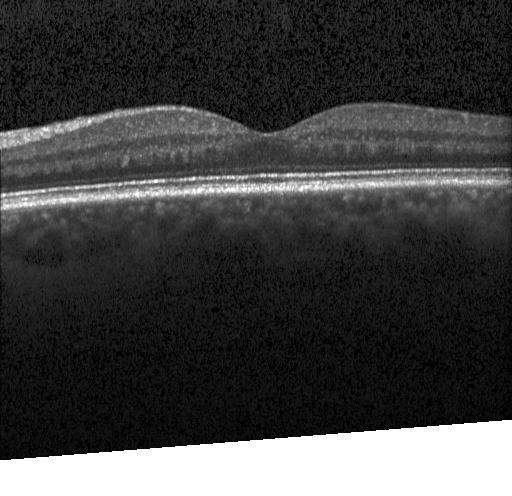
Spectral-domain OCT, OCT line scan — This B-scan demonstrates no CNV, no DME, and no drusen.